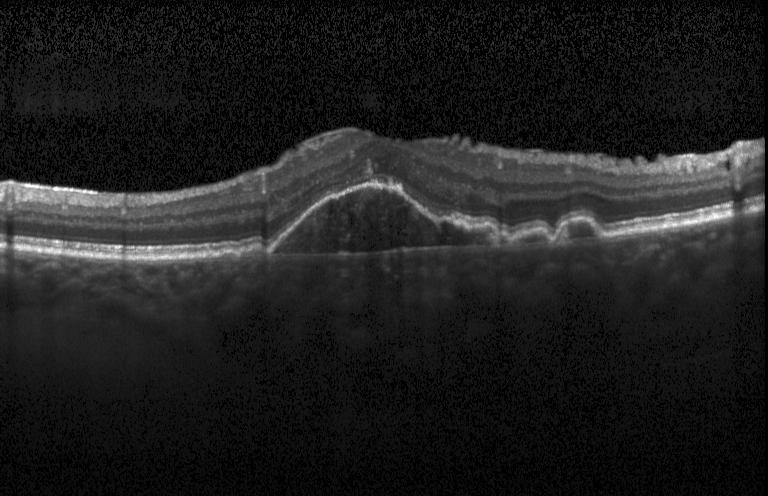
OCT line scan, acquired on a Heidelberg Spectralis
Macular OCT: a choroidal neovascular membrane.